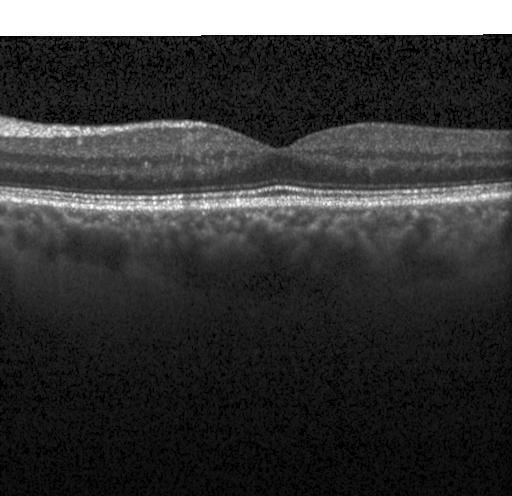 OCT line scan · horizontal scan through the fovea · Heidelberg Spectralis — The scan shows no choroidal neovascularization, diabetic macular edema, or drusen.